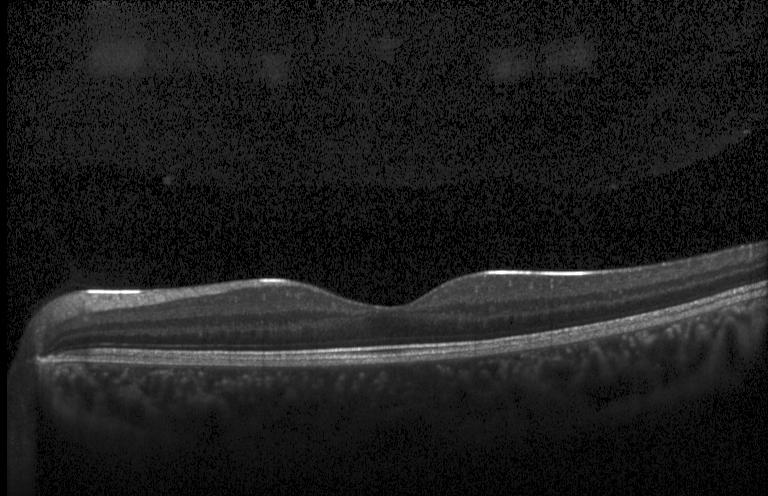

Finding: no choroidal neovascularization, no diabetic macular edema, and no drusen.